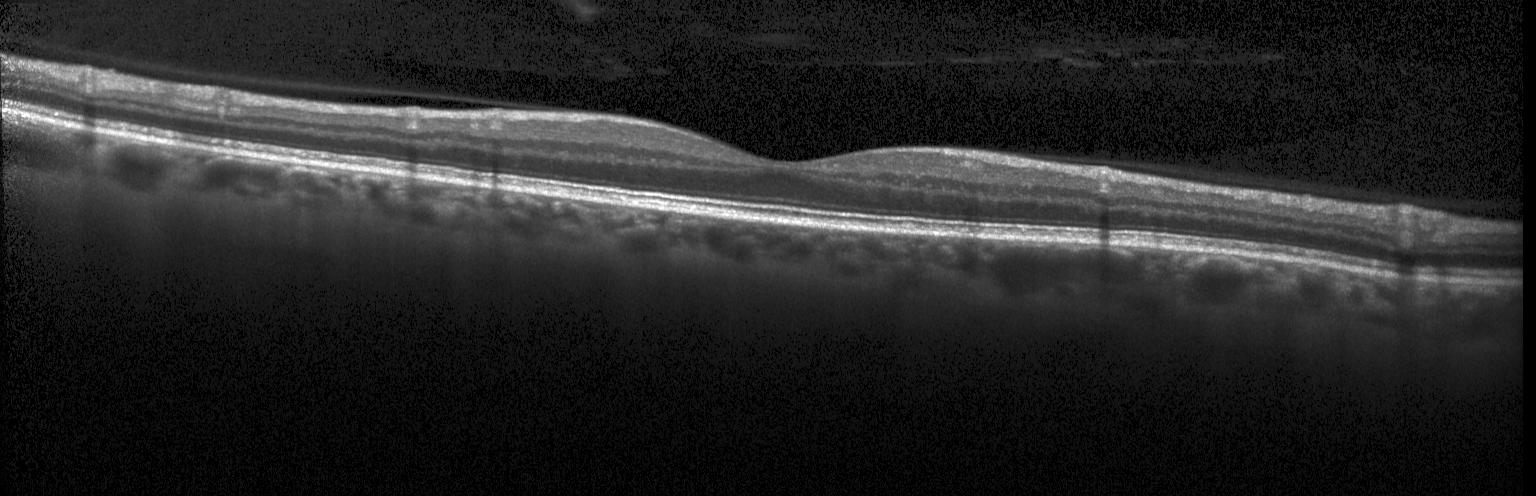 OCT B-scan showing neither choroidal neovascularization, diabetic macular edema, nor drusen.